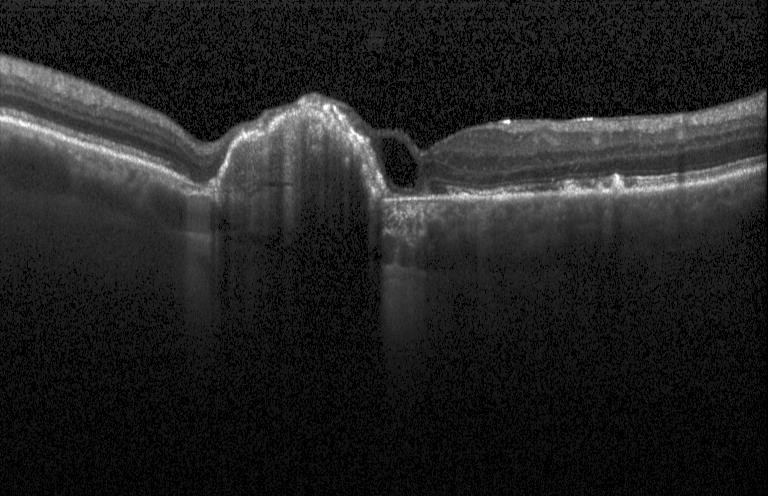

Retinal OCT cross-section. SD-OCT. Heidelberg Spectralis OCT system. Through the macula — The scan shows choroidal neovascularization.